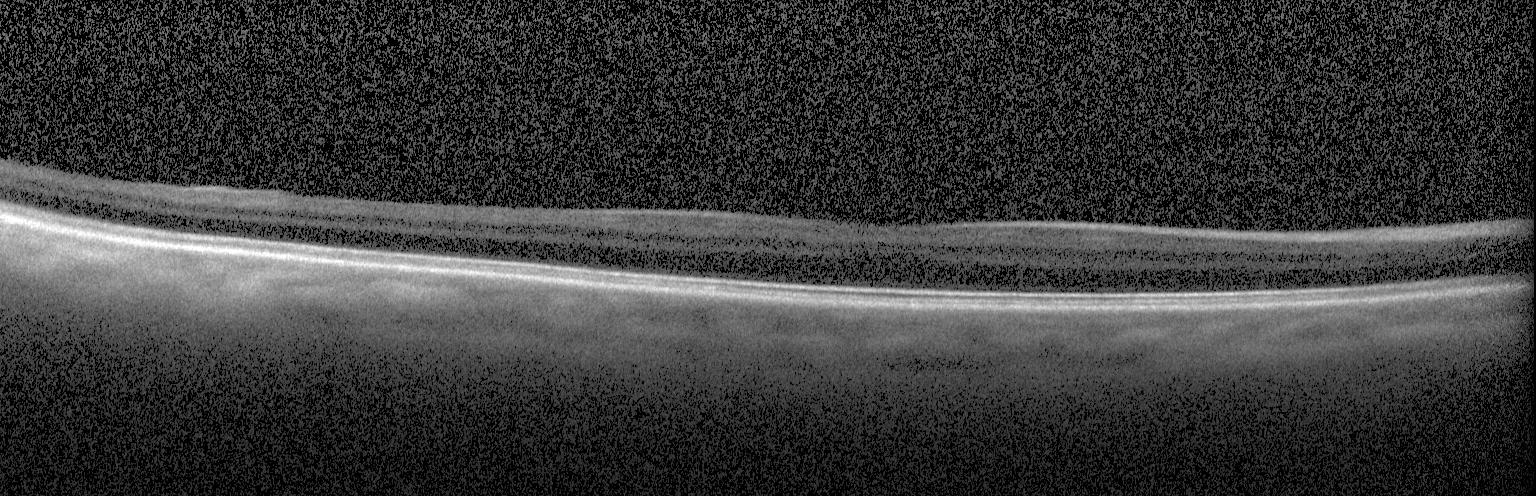 Diagnosis: no CNV, DME, or drusen.